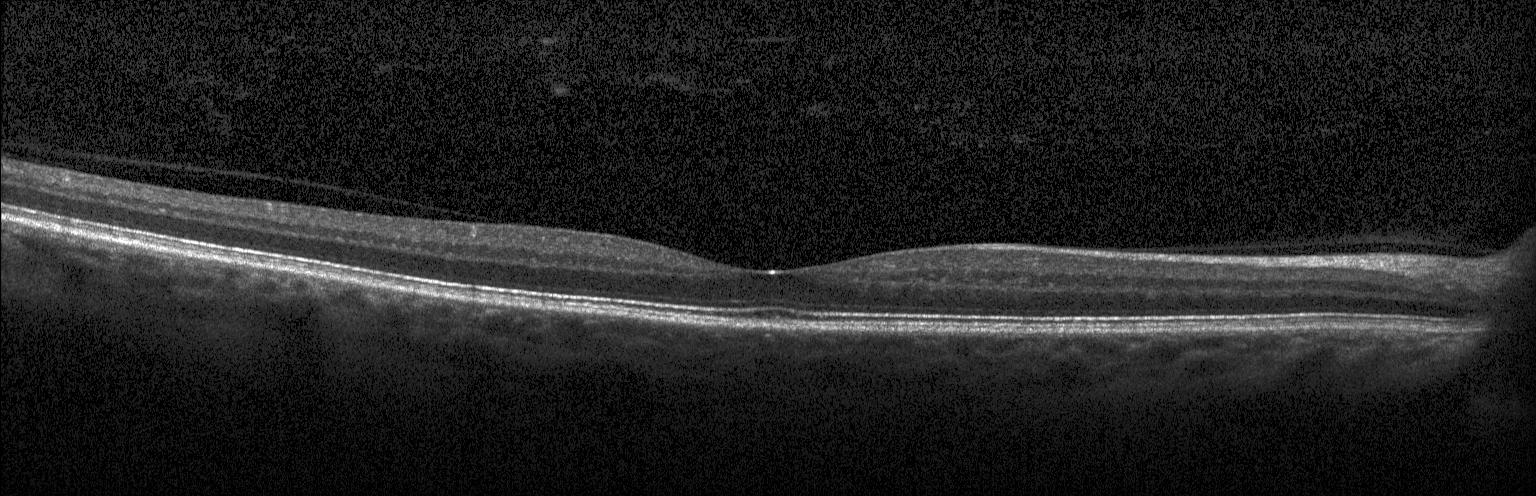
Spectral-domain optical coherence tomography · acquired on a Heidelberg Spectralis · macular scan · optical coherence tomography B-scan. OCT finding: no CNV, no DME, and no drusen.